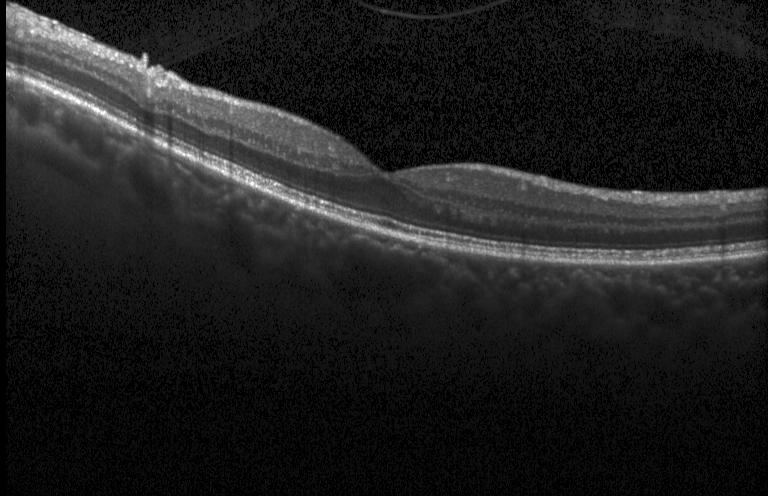 The scan shows neither choroidal neovascularization, diabetic macular edema, nor drusen.